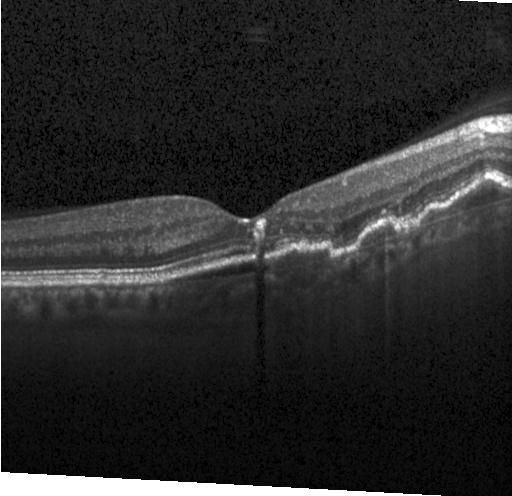
Heidelberg Spectralis OCT system; macular scan; OCT B-scan; spectral-domain optical coherence tomography
Diagnosis: a choroidal neovascular membrane.